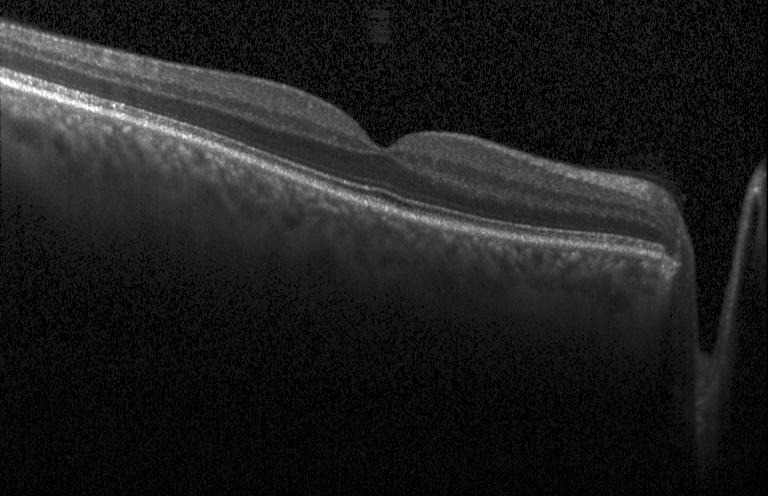

Optical coherence tomography scan. Dx: no choroidal neovascularization, no diabetic macular edema, and no drusen.